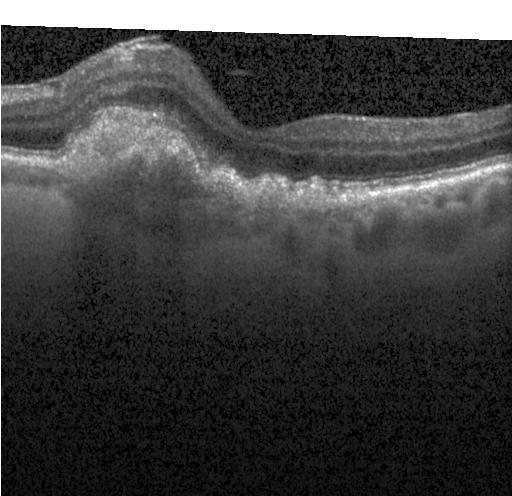
Impression: a choroidal neovascular membrane.